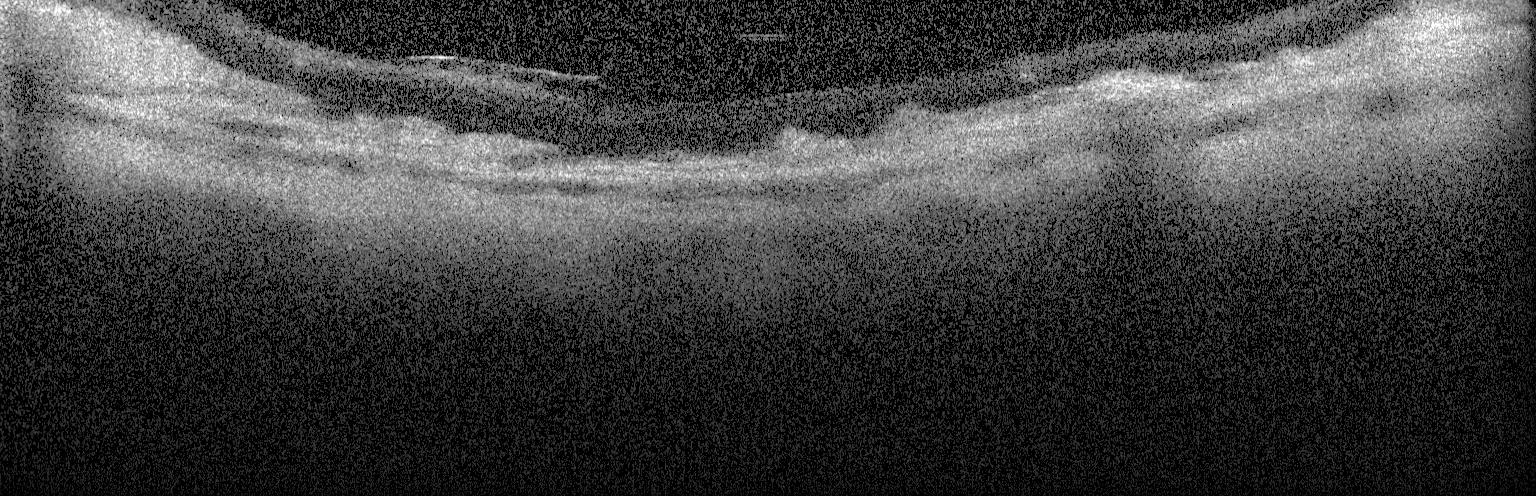 Macular OCT demonstrating choroidal neovascularization (CNV).